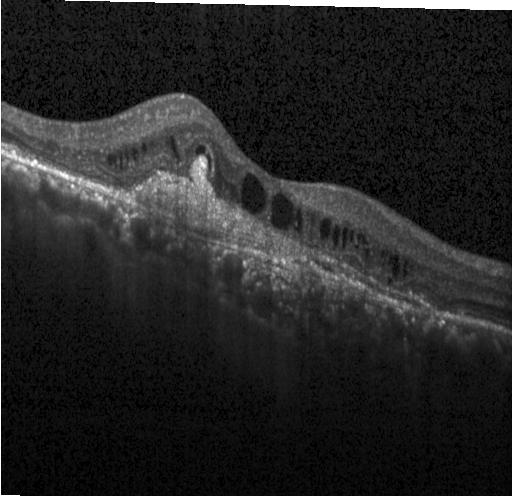 Assessment: a choroidal neovascular membrane.